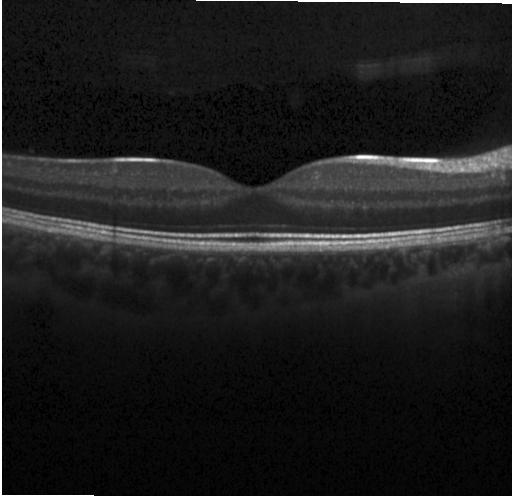
Heidelberg Spectralis OCT system, through the macula, retinal OCT cross-section, spectral-domain OCT — Diagnosis: neither CNV, DME, nor drusen.